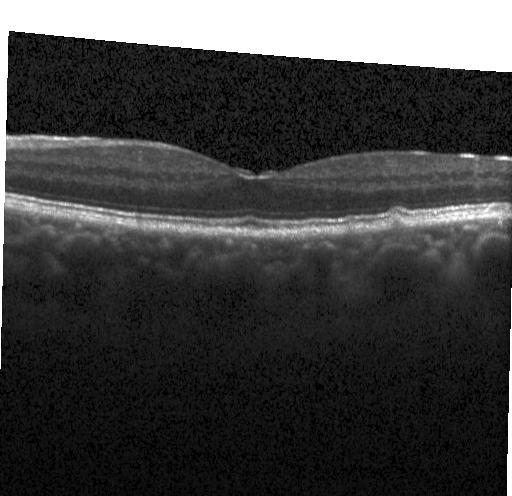

Retinal OCT B-scan.
Impression: multiple drusen.